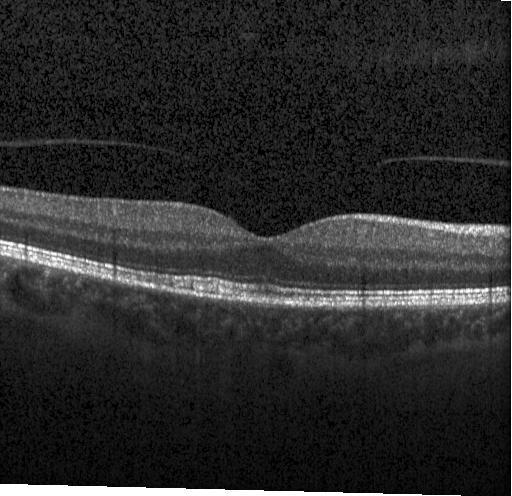
Retinal OCT cross-section; macular scan
OCT finding: neither CNV, DME, nor drusen.